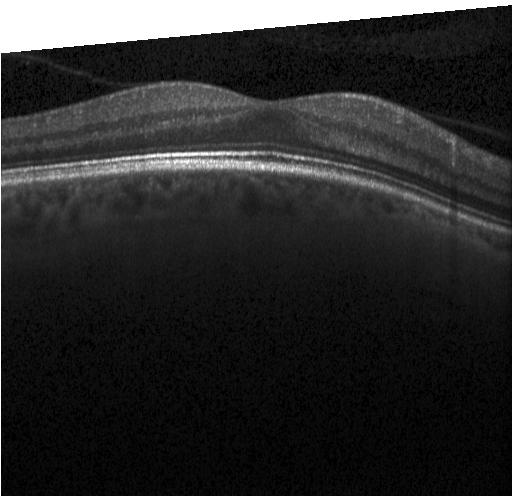
Acquired on a Heidelberg Spectralis, centered on the fovea, optical coherence tomography scan — Diagnosis: no choroidal neovascularization, no diabetic macular edema, and no drusen.